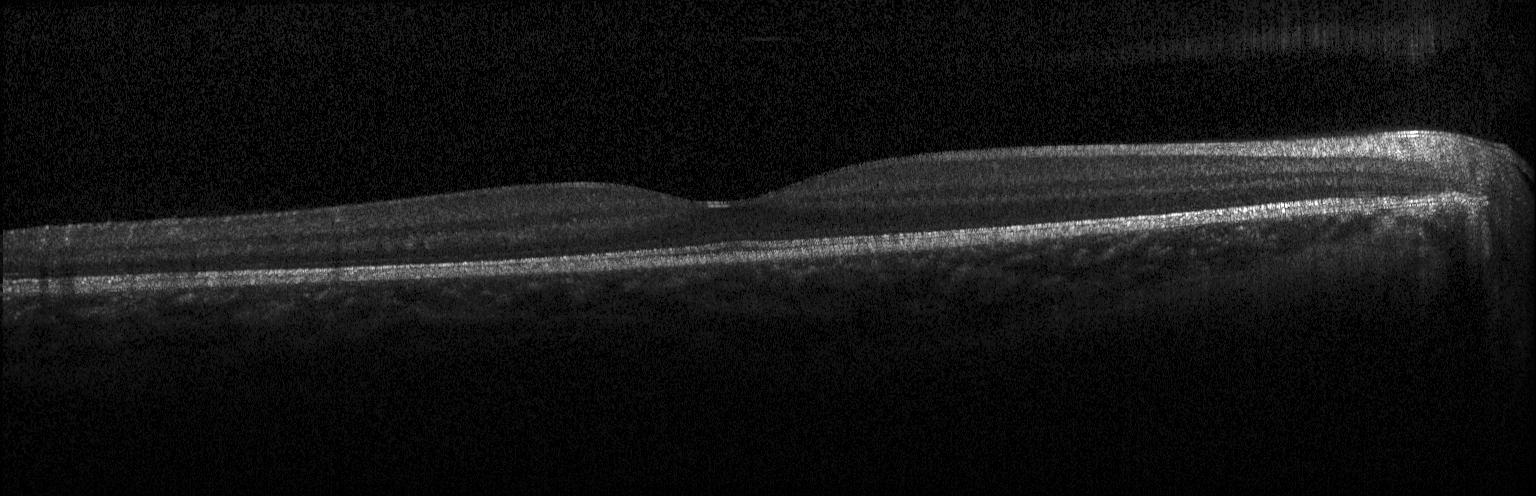 Optical coherence tomography B-scan — The scan shows no choroidal neovascularization, diabetic macular edema, or drusen.